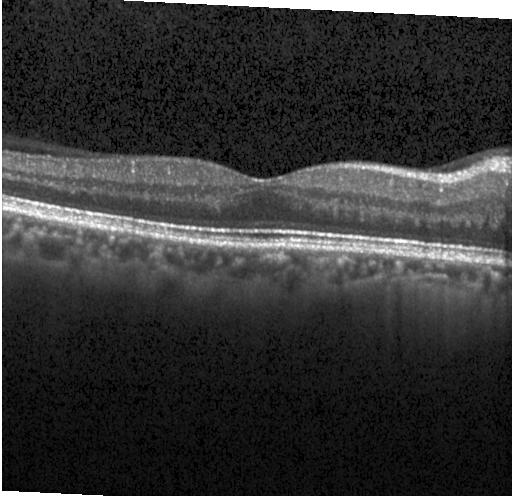

Diagnosis: no choroidal neovascularization, no diabetic macular edema, and no drusen.